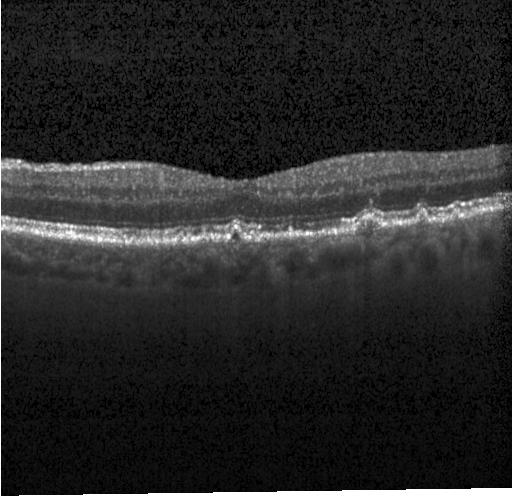 Macular OCT demonstrating sub-RPE drusenoid deposits.